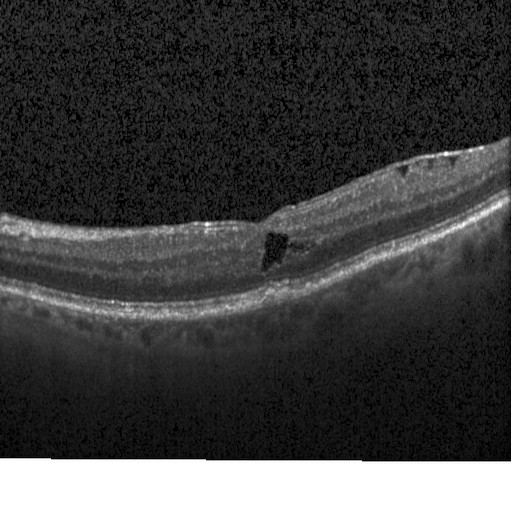

SD-OCT. Retinal OCT B-scan. Horizontal scan through the fovea — Impression: diabetic macular edema.